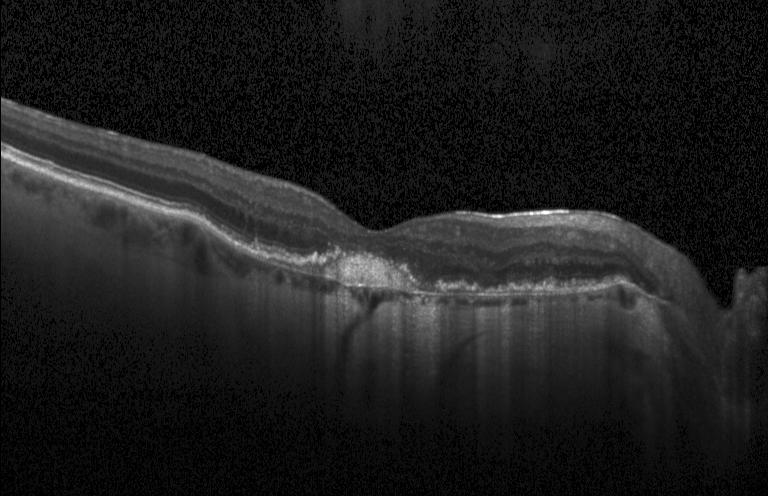

Diagnosis: a choroidal neovascular membrane.